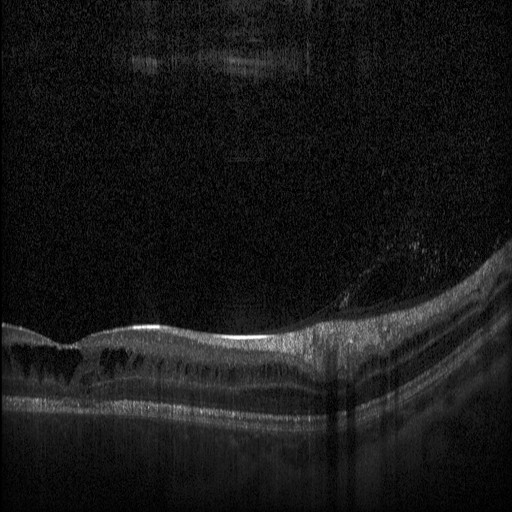

OCT B-scan · fovea-centered · acquired on a Heidelberg Spectralis
The scan shows diabetic macular edema (DME).